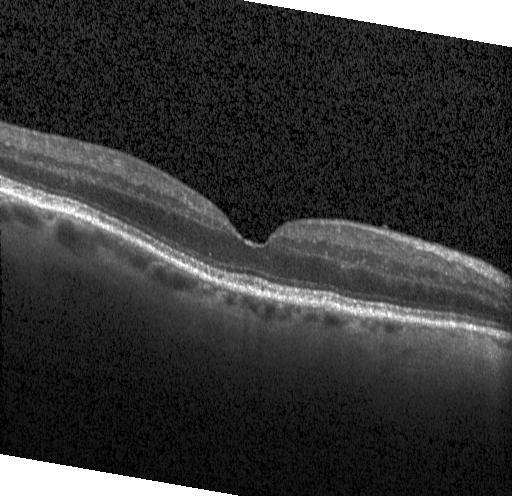

Finding: neither choroidal neovascularization, diabetic macular edema, nor drusen.